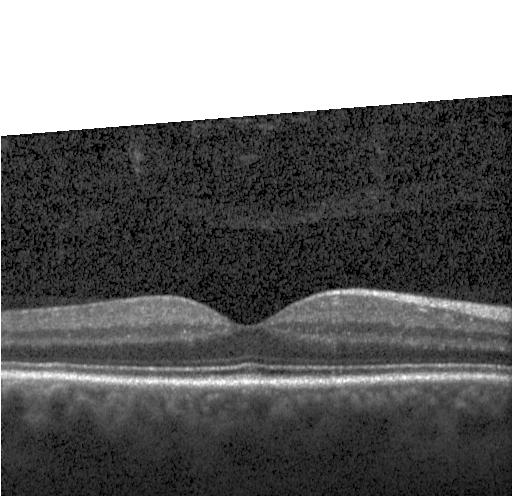
Spectral-domain OCT B-scan: no evidence of choroidal neovascularization, diabetic macular edema, or drusen.